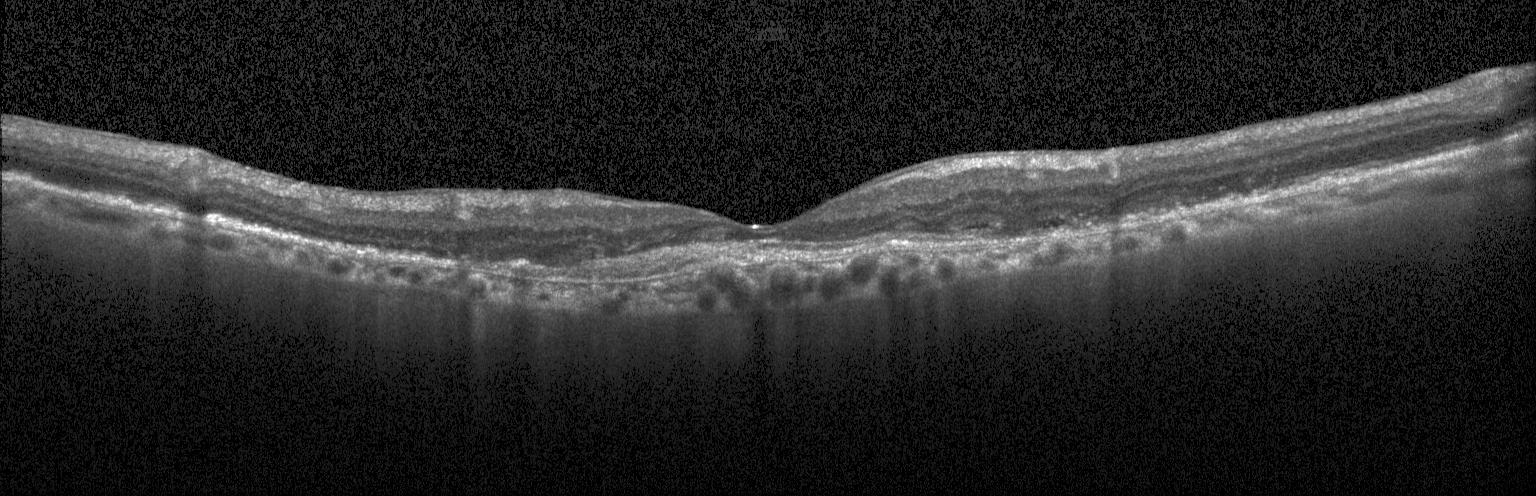

Choroidal neovascularization (CNV).